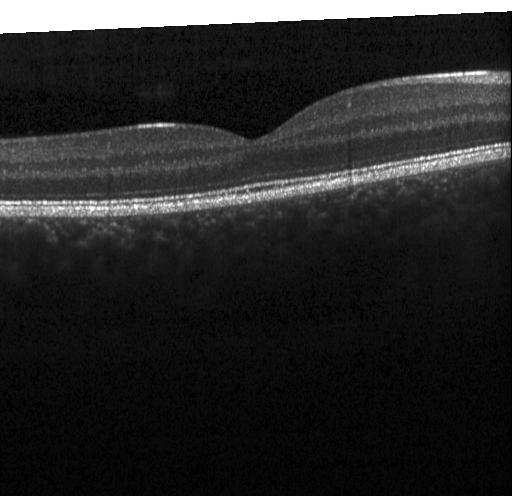

No choroidal neovascularization, no diabetic macular edema, and no drusen.